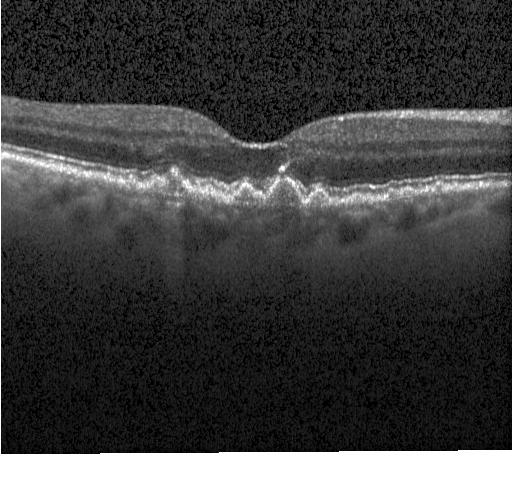 Retinal OCT cross-section showing drusen.